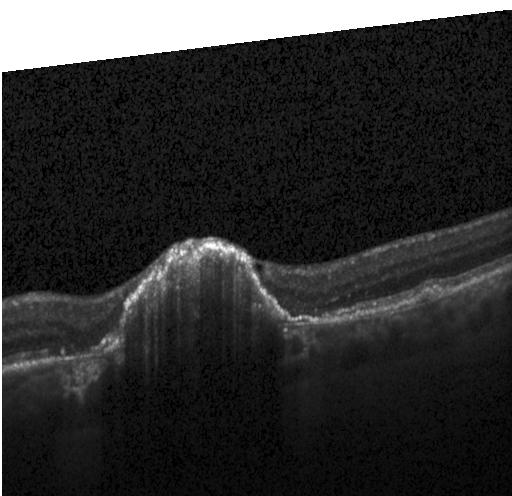 Dx: a choroidal neovascular membrane.